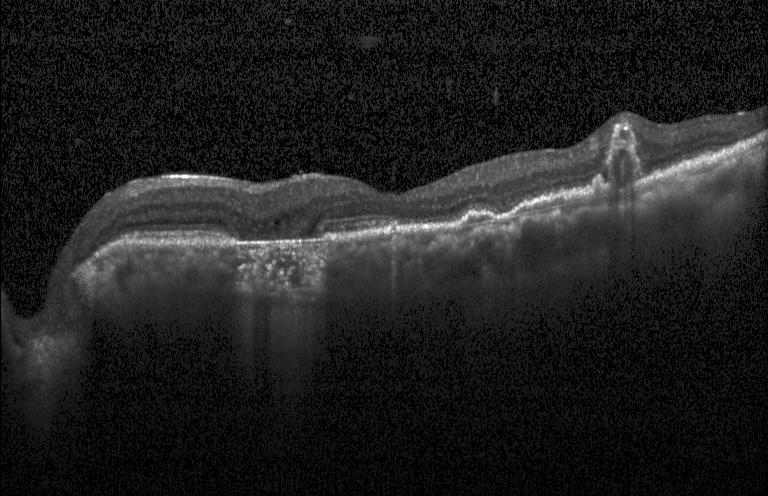
Acquired on a Heidelberg Spectralis · through the macula · retinal OCT B-scan · spectral-domain optical coherence tomography — Impression: a choroidal neovascular membrane.